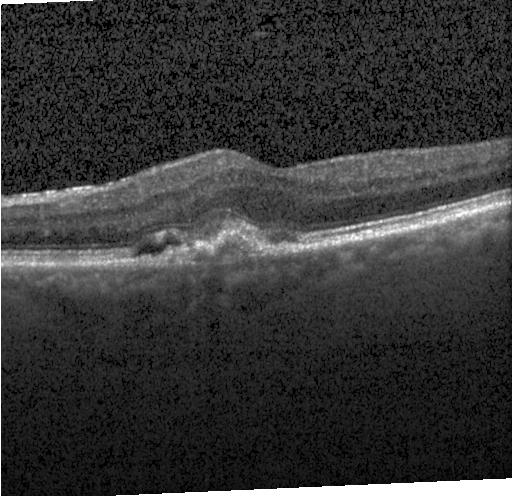

Finding: CNV.